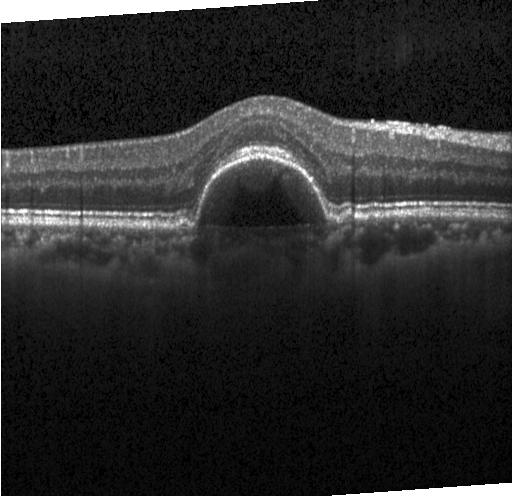
Finding: a choroidal neovascular membrane.